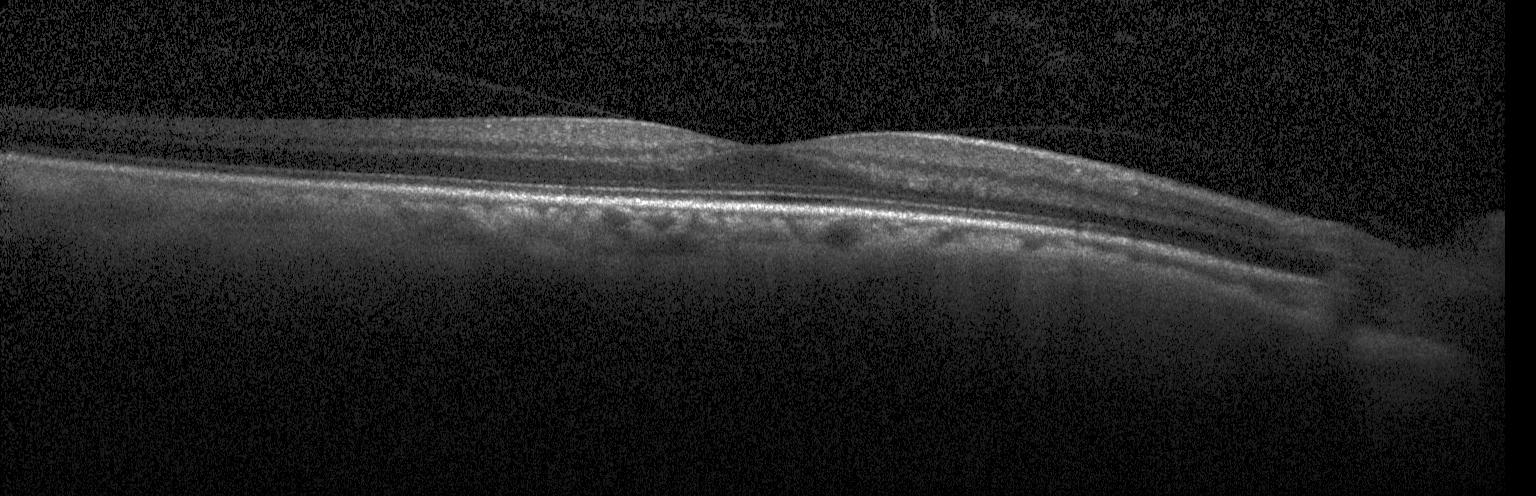 OCT line scan — Impression: no choroidal neovascularization, no diabetic macular edema, and no drusen.